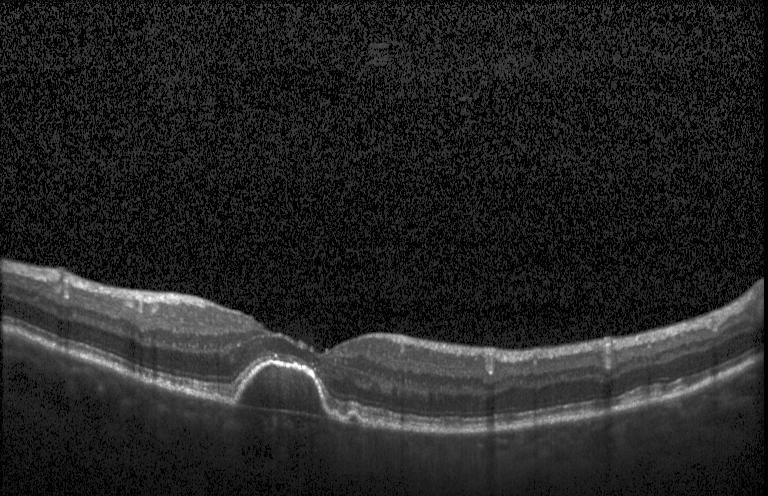
Retinal OCT cross-section showing choroidal neovascularization (CNV).